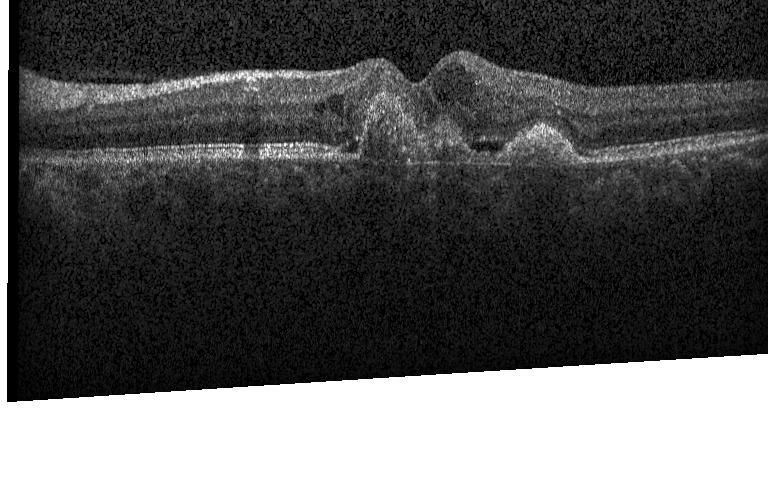 OCT scan showing a choroidal neovascular membrane.